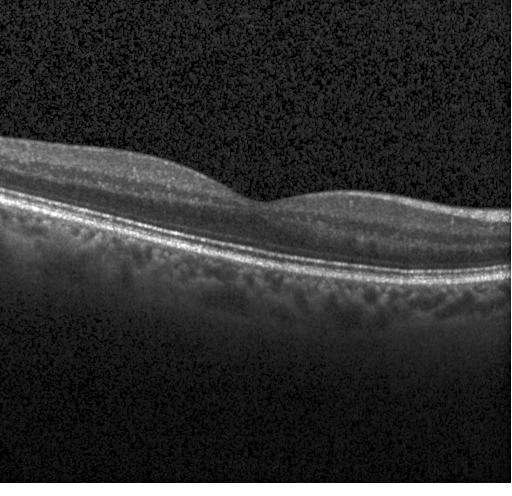

Retinal OCT cross-section
The scan shows no CNV, no DME, and no drusen.